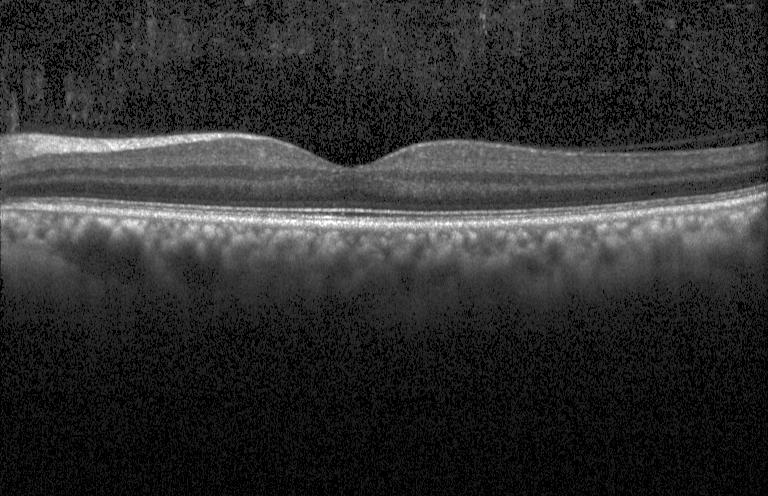 The scan shows no CNV, DME, or drusen.